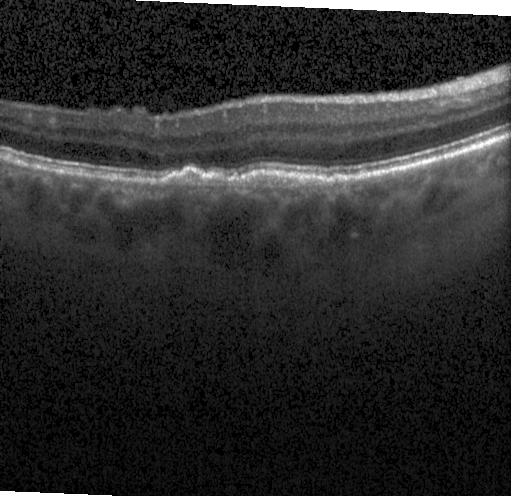
SD-OCT; instrument: Heidelberg Spectralis; optical coherence tomography scan; centered on the fovea.
Dx: choroidal neovascularization (CNV).